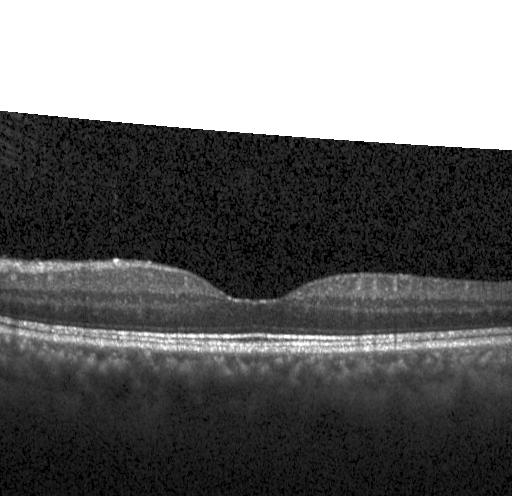 Finding: no CNV, no DME, and no drusen.